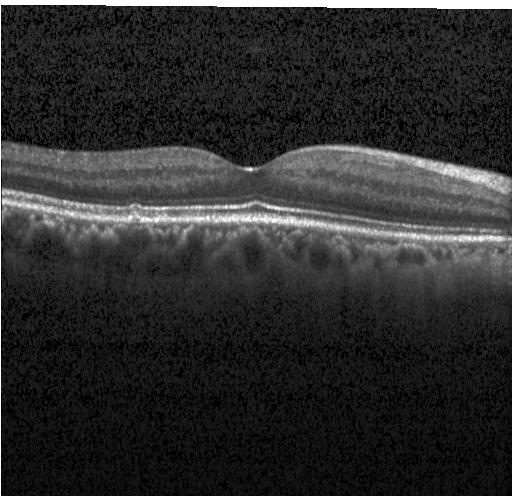 Optical coherence tomography B-scan
OCT finding: sub-RPE drusenoid deposits.